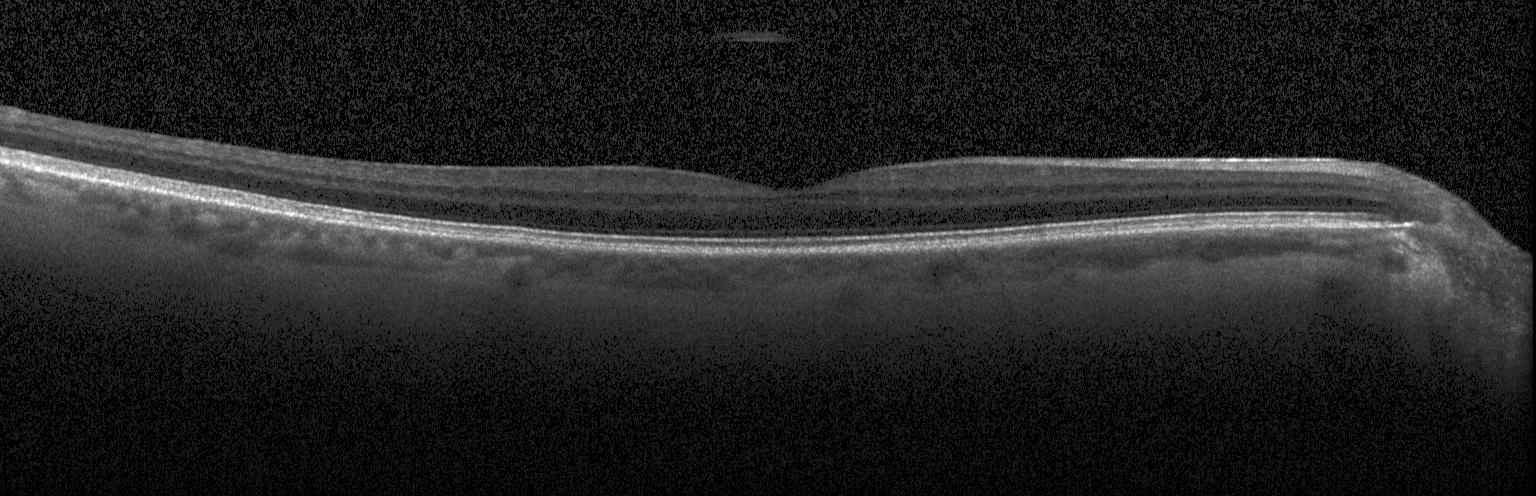
Macular scan · instrument: Heidelberg Spectralis · OCT B-scan. OCT finding: no choroidal neovascularization, no diabetic macular edema, and no drusen.